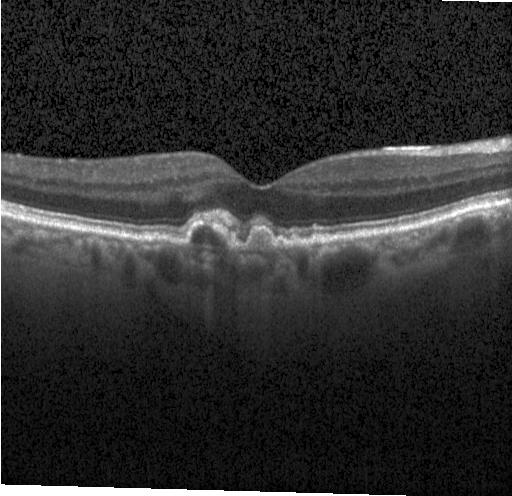
The scan shows CNV.